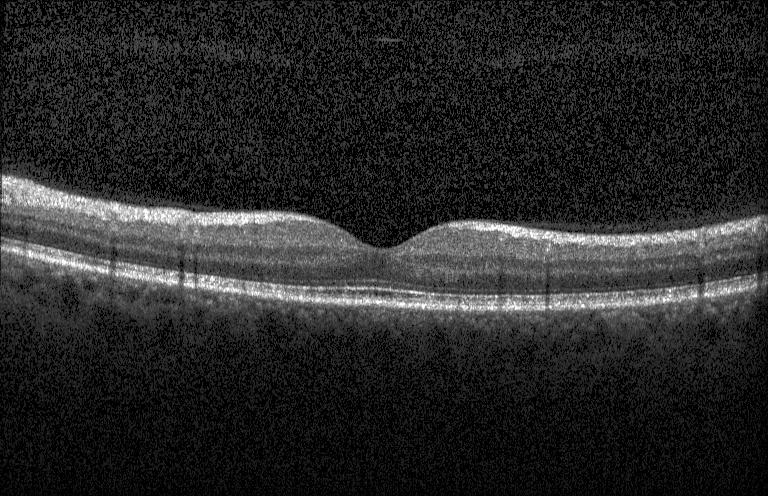

Instrument: Heidelberg Spectralis, horizontal scan through the fovea, optical coherence tomography B-scan — The scan shows no choroidal neovascularization, no diabetic macular edema, and no drusen.